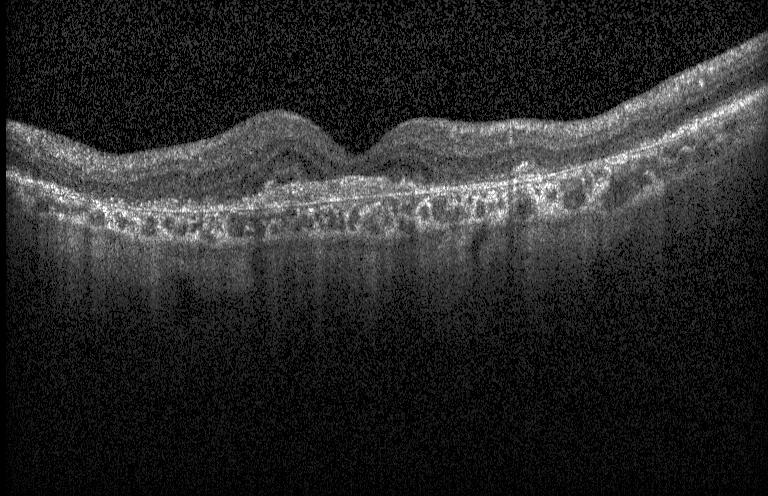
Spectral-domain optical coherence tomography; optical coherence tomography B-scan; centered on the fovea. The scan shows choroidal neovascularization (CNV).